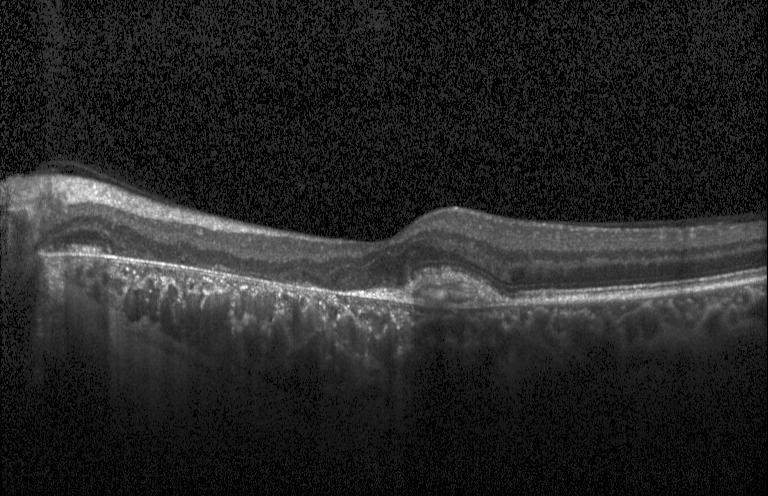
Macular OCT: a choroidal neovascular membrane.